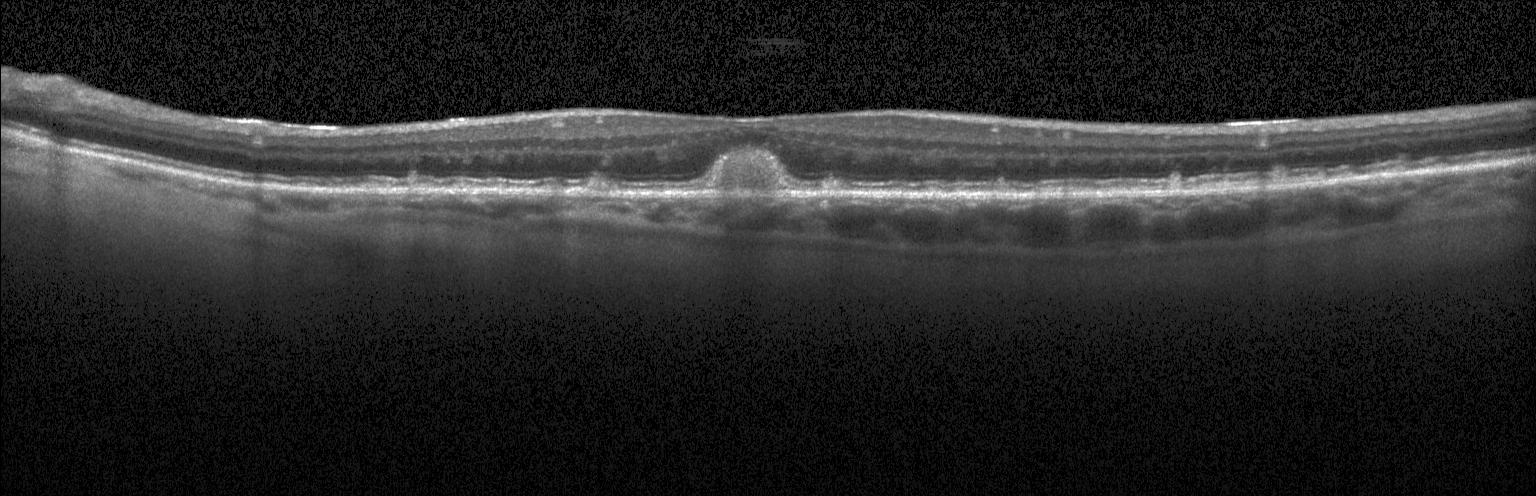

Spectral-domain OCT B-scan: a choroidal neovascular membrane.